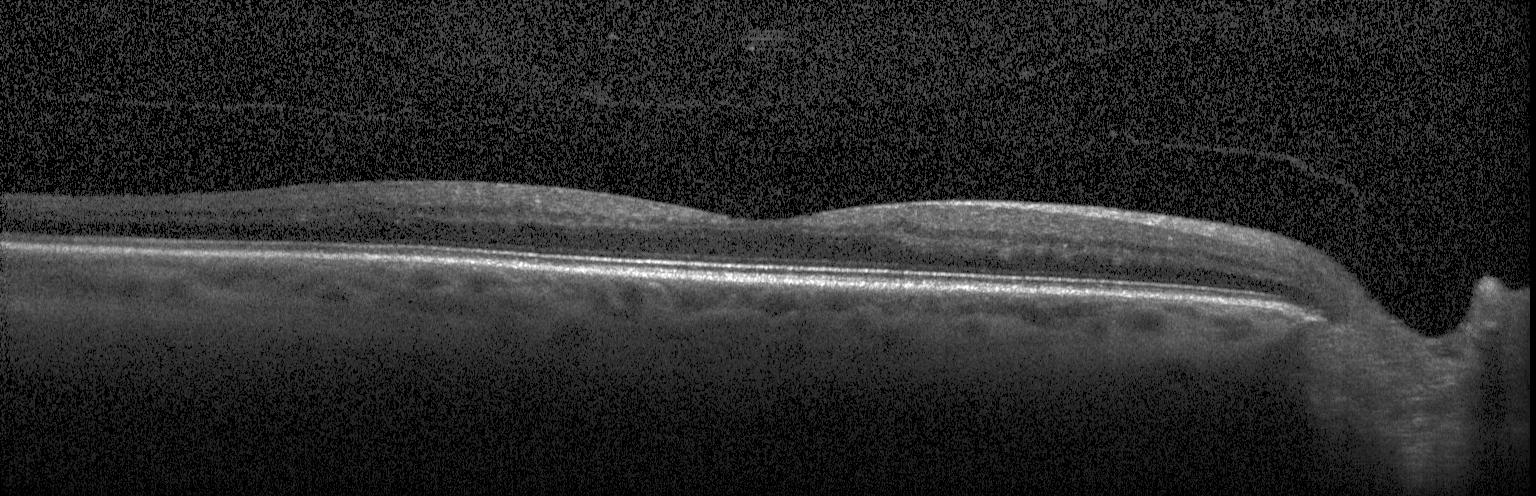 Finding: no choroidal neovascularization, diabetic macular edema, or drusen.